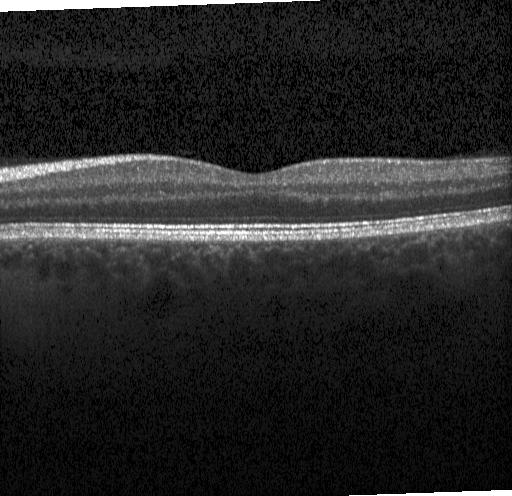

Impression: neither choroidal neovascularization, diabetic macular edema, nor drusen.